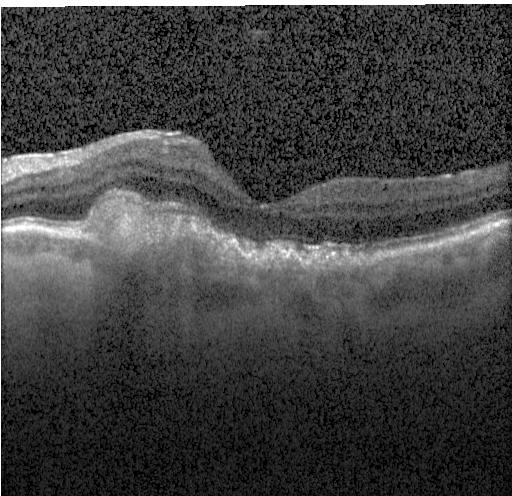

OCT line scan. Impression: a choroidal neovascular membrane.